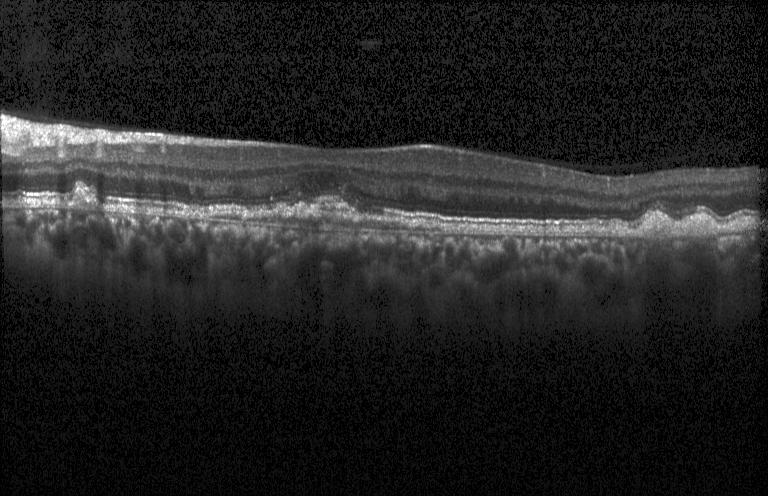 Macular OCT: choroidal neovascularization.